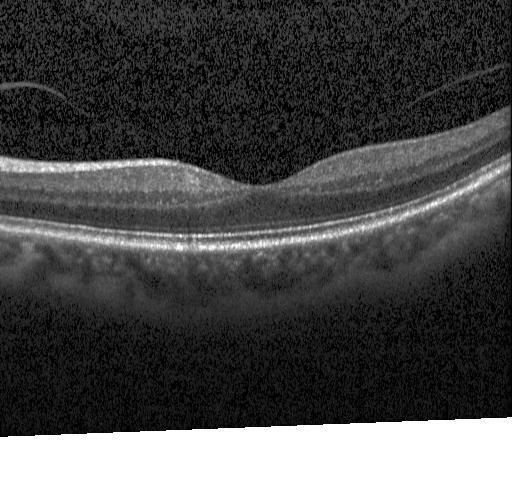 Dx: no CNV, no DME, and no drusen.